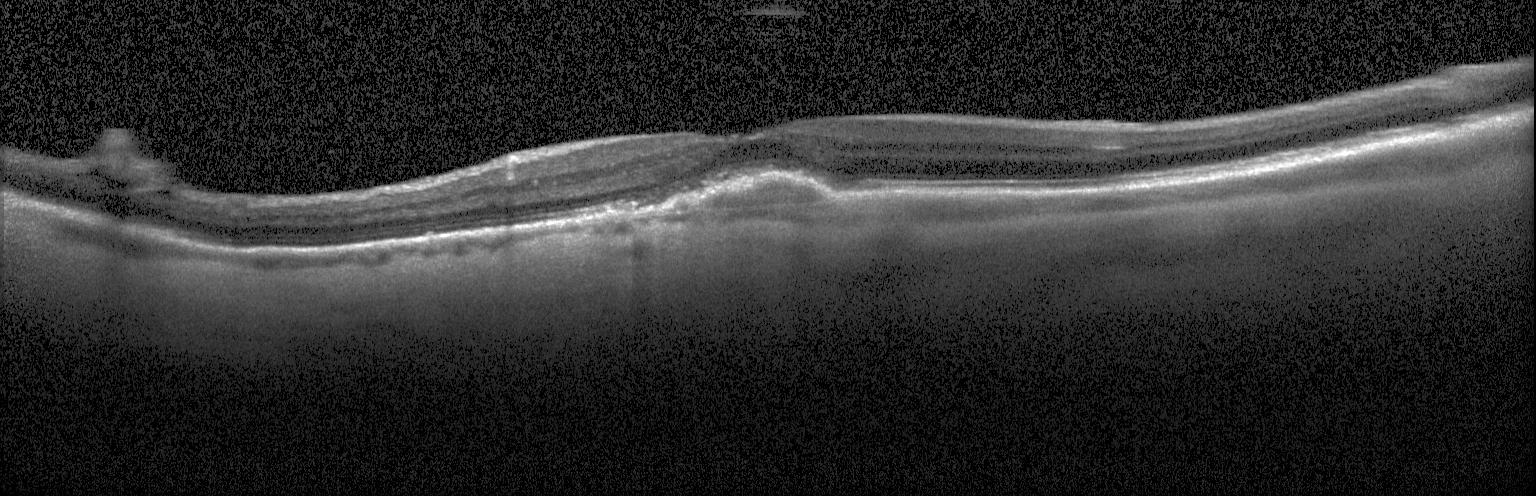 Macular scan. Retinal OCT cross-section. SD-OCT. Heidelberg Spectralis.
Macular OCT: a choroidal neovascular membrane.